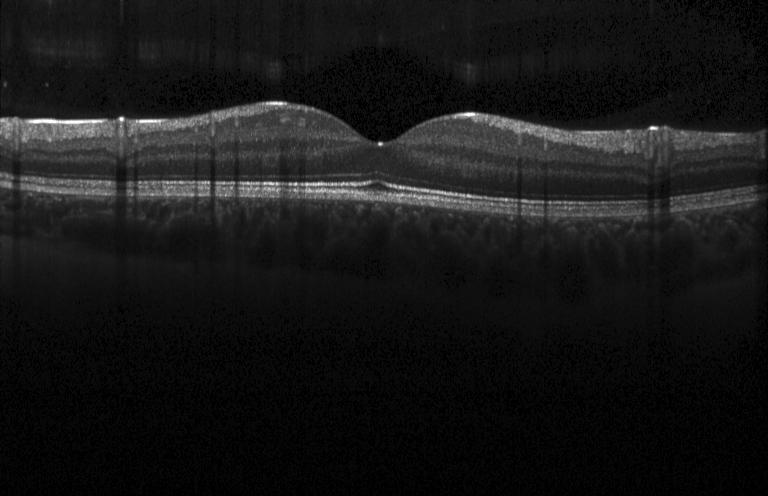 OCT scan showing neither choroidal neovascularization, diabetic macular edema, nor drusen.